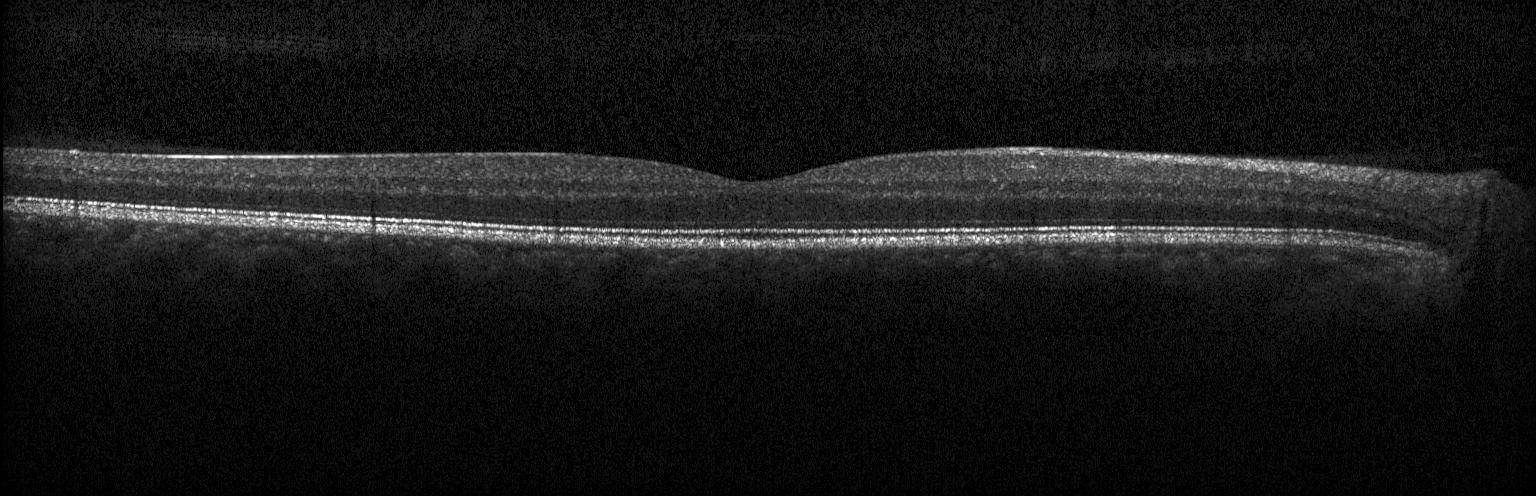
Spectral-domain OCT, Heidelberg Spectralis OCT system, through the macula, OCT line scan.
Impression: no choroidal neovascularization, diabetic macular edema, or drusen.